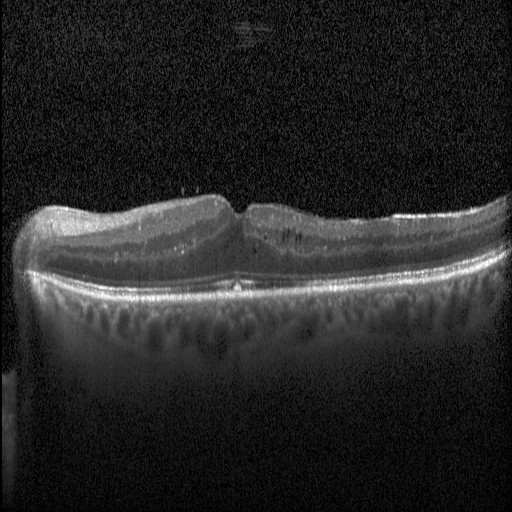 Through the macula, spectral-domain optical coherence tomography, retinal OCT B-scan.
This B-scan demonstrates DME.